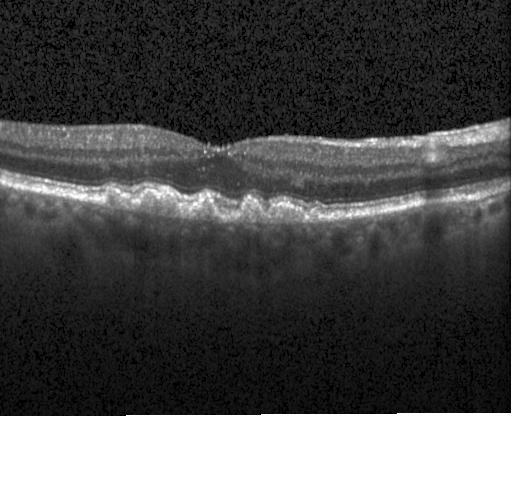 Retinal OCT cross-section. Impression: drusen.